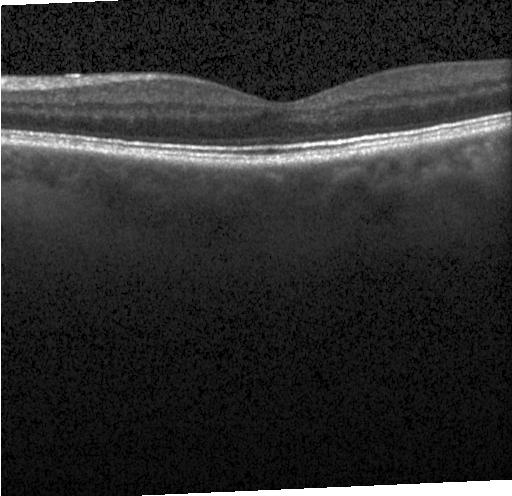
OCT B-scan; macular scan; acquired on a Heidelberg Spectralis; spectral-domain optical coherence tomography — Macular OCT: no choroidal neovascularization, no diabetic macular edema, and no drusen.